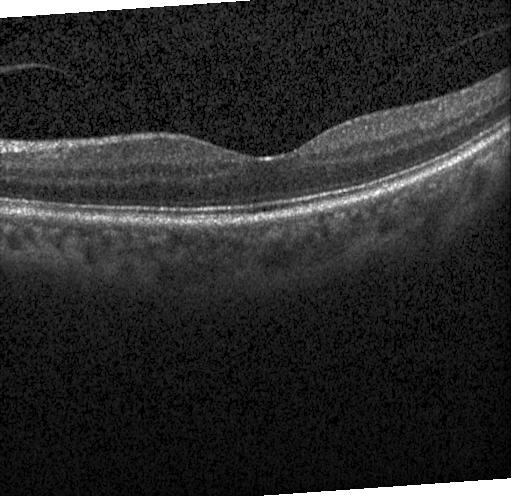
OCT line scan. Fovea-centered
No choroidal neovascularization, no diabetic macular edema, and no drusen.